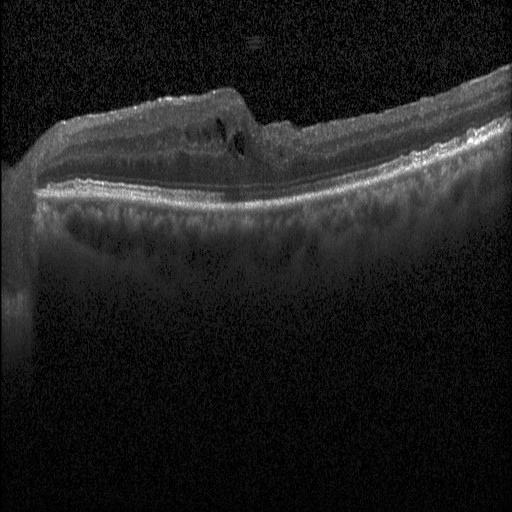 Retinal OCT cross-section. Macular OCT: diabetic macular edema (DME).